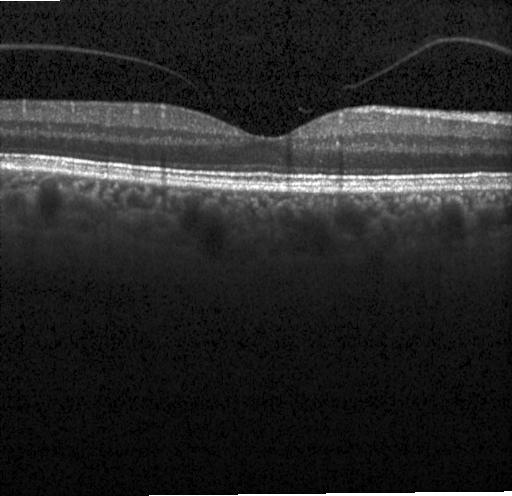
Optical coherence tomography scan
This B-scan demonstrates no choroidal neovascularization, no diabetic macular edema, and no drusen.